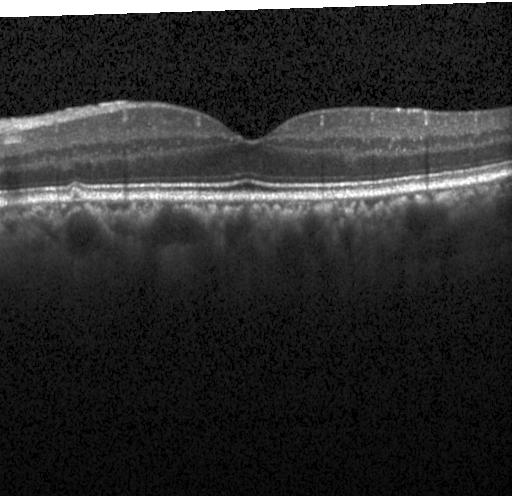
OCT B-scan; spectral-domain optical coherence tomography — Dx: sub-RPE drusenoid deposits.